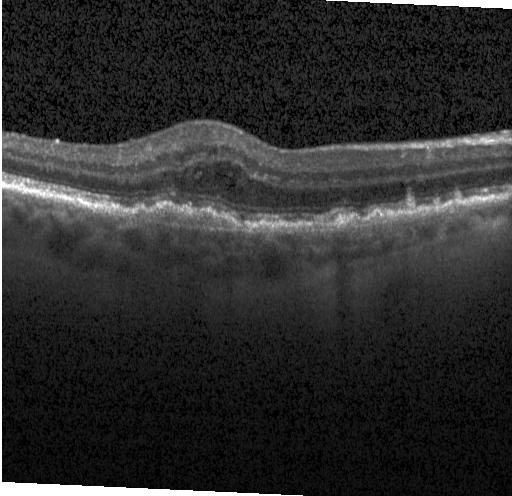 Macular OCT: a choroidal neovascular membrane.